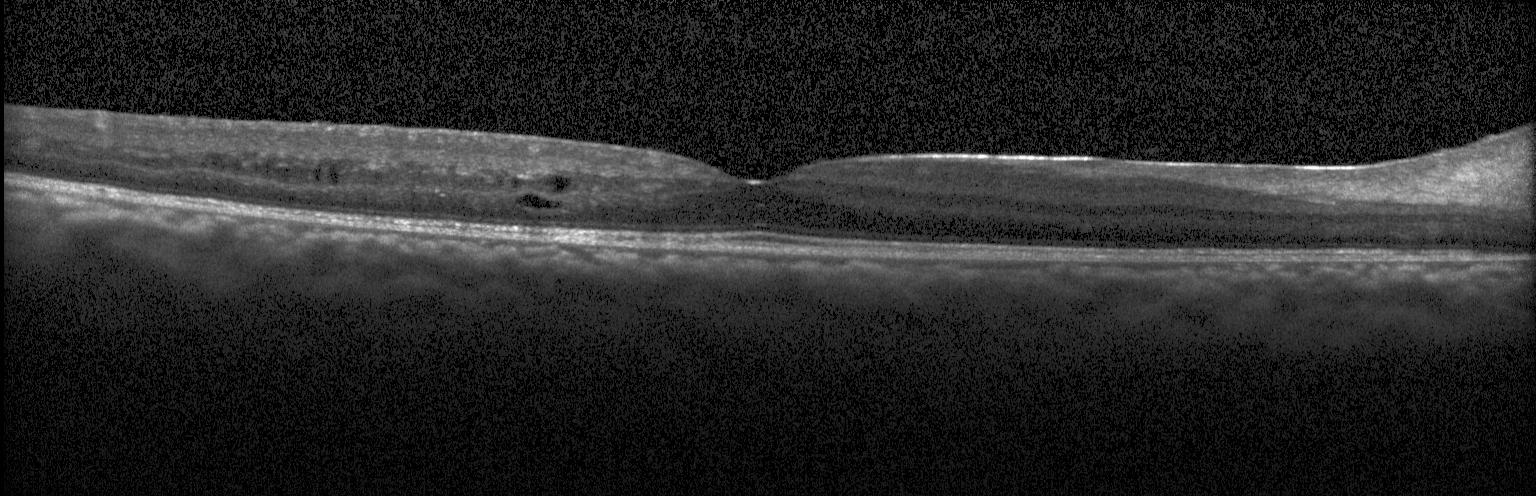 Diabetic macular edema (DME).